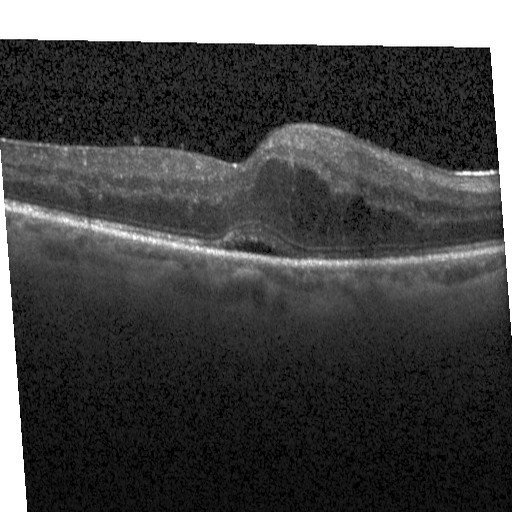
OCT finding: diabetic macular edema.